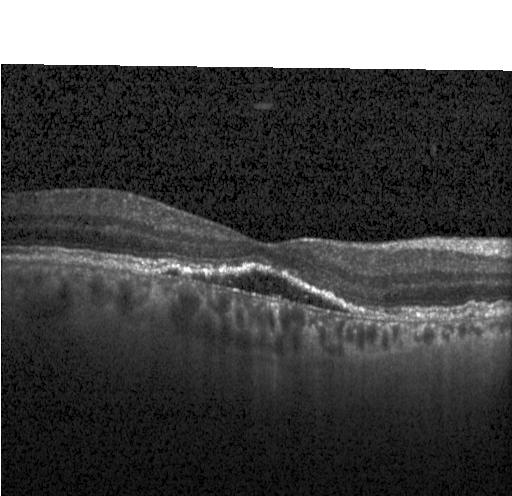
OCT finding: choroidal neovascularization (CNV).